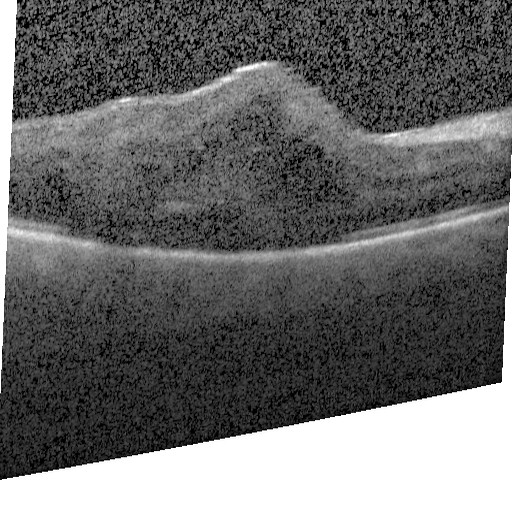

Optical coherence tomography B-scan. OCT finding: DME.